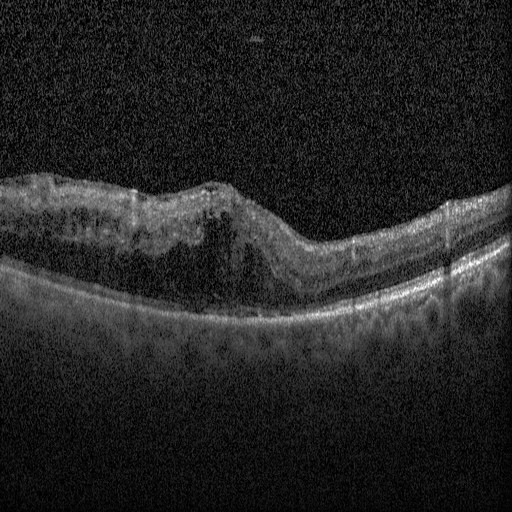

OCT B-scan. Dx: DME.